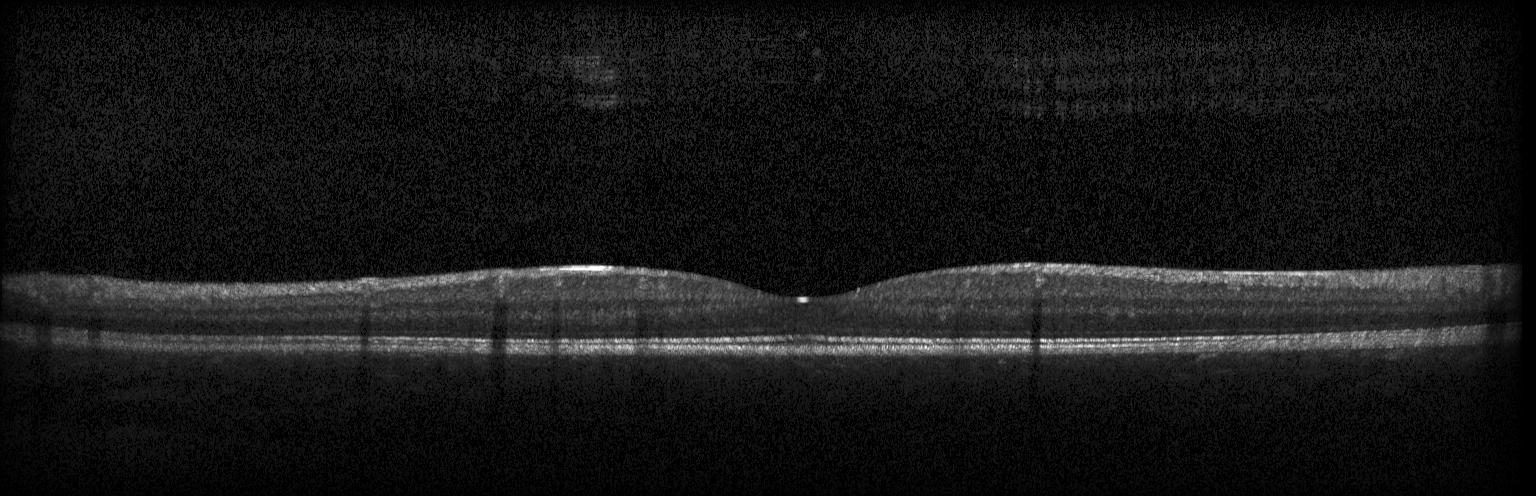 OCT line scan — Dx: neither choroidal neovascularization, diabetic macular edema, nor drusen.